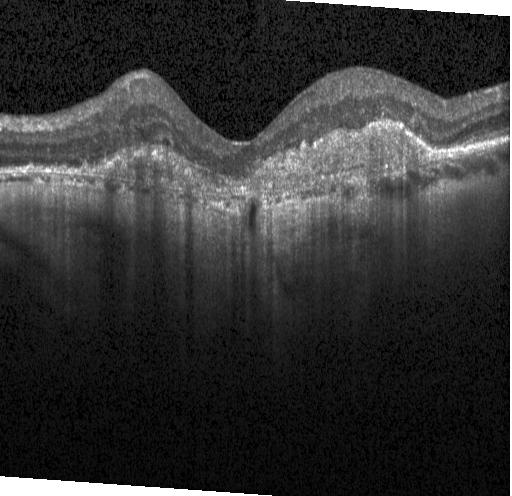
Macular OCT: a choroidal neovascular membrane.